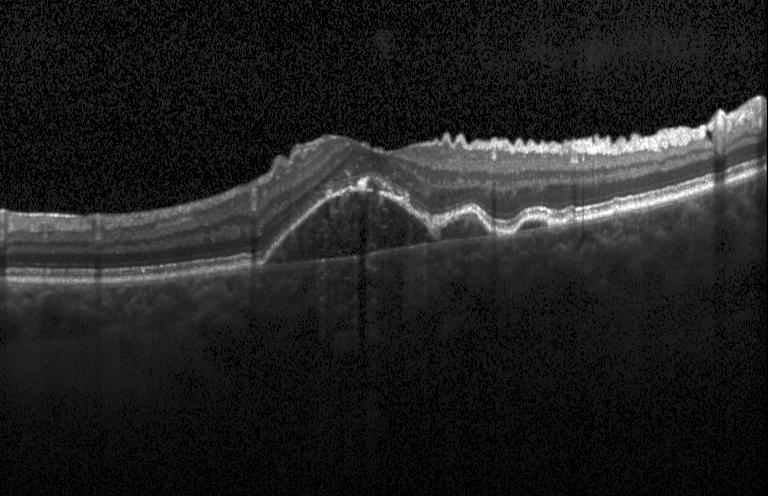
Spectral-domain optical coherence tomography, macular scan, optical coherence tomography B-scan.
Diagnosis: choroidal neovascularization (CNV).